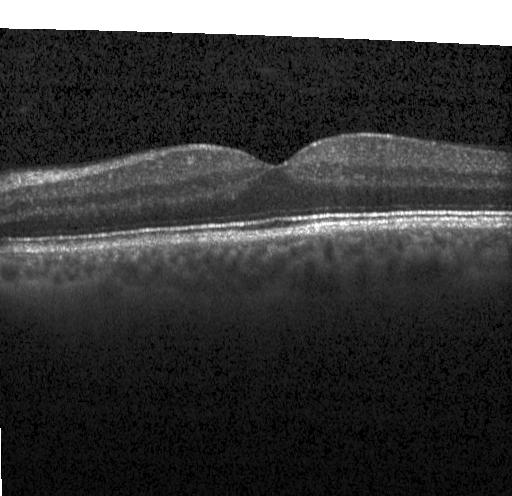

Dx: no choroidal neovascularization, no diabetic macular edema, and no drusen.